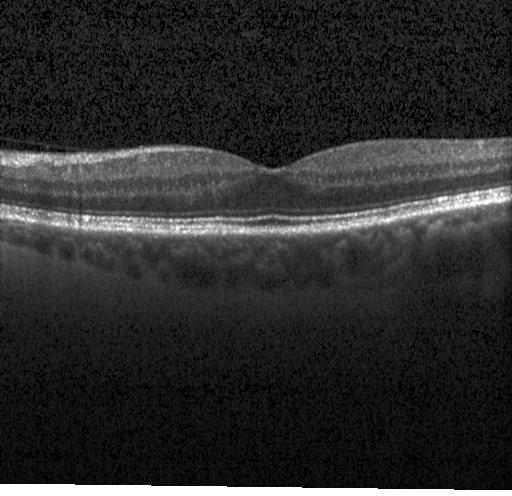 Acquired on a Heidelberg Spectralis; retinal OCT B-scan; SD-OCT; through the macula — The scan shows neither CNV, DME, nor drusen.